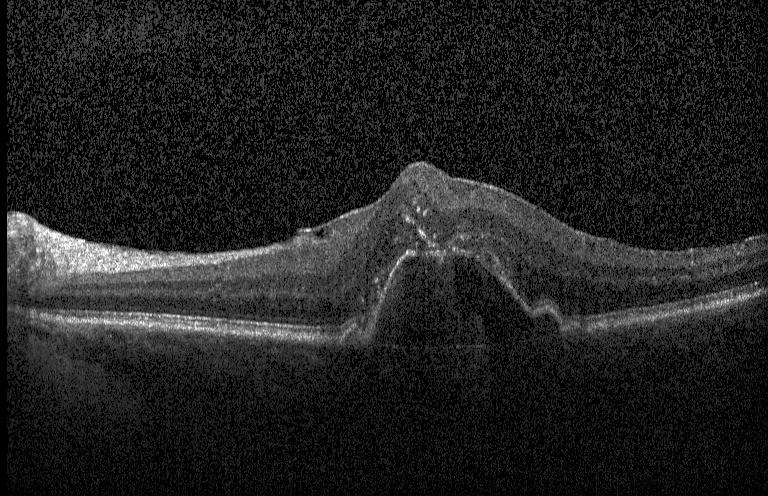 Optical coherence tomography B-scan — Macular OCT: a choroidal neovascular membrane.